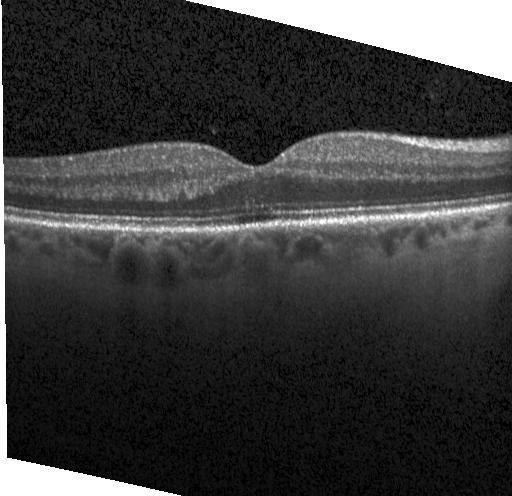

Acquired on a Heidelberg Spectralis. OCT line scan
The scan shows no choroidal neovascularization, diabetic macular edema, or drusen.